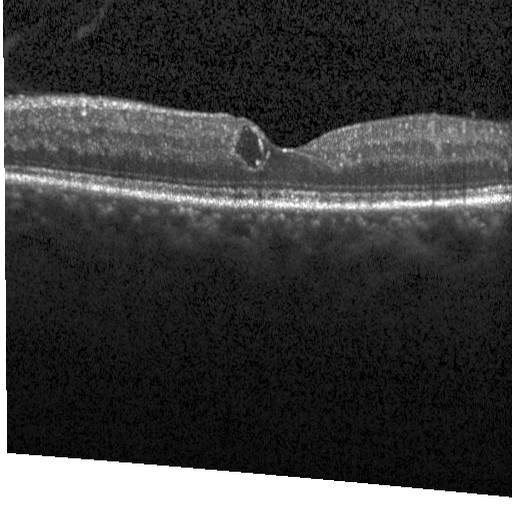 Spectral-domain OCT, through the macula, Heidelberg Spectralis, optical coherence tomography B-scan — Dx: DME.